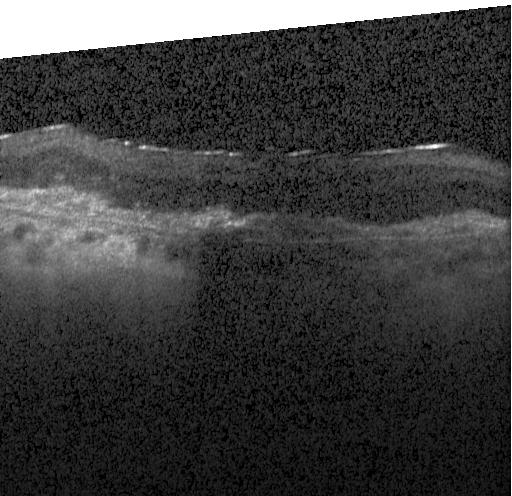

OCT line scan.
Diagnosis: CNV.